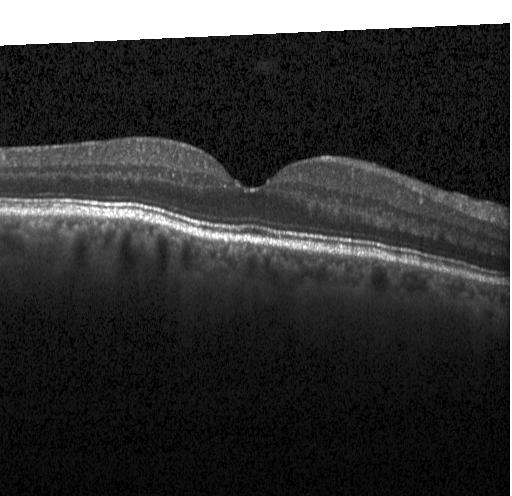 Instrument: Heidelberg Spectralis; optical coherence tomography scan; centered on the fovea; SD-OCT. Finding: no choroidal neovascularization, no diabetic macular edema, and no drusen.